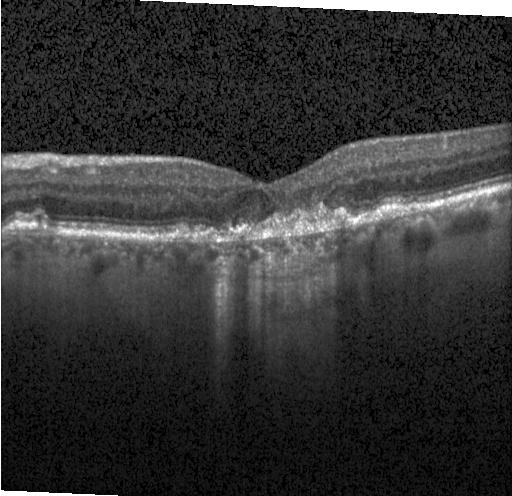 Optical coherence tomography scan. Through the macula. Heidelberg Spectralis. Finding: a choroidal neovascular membrane.